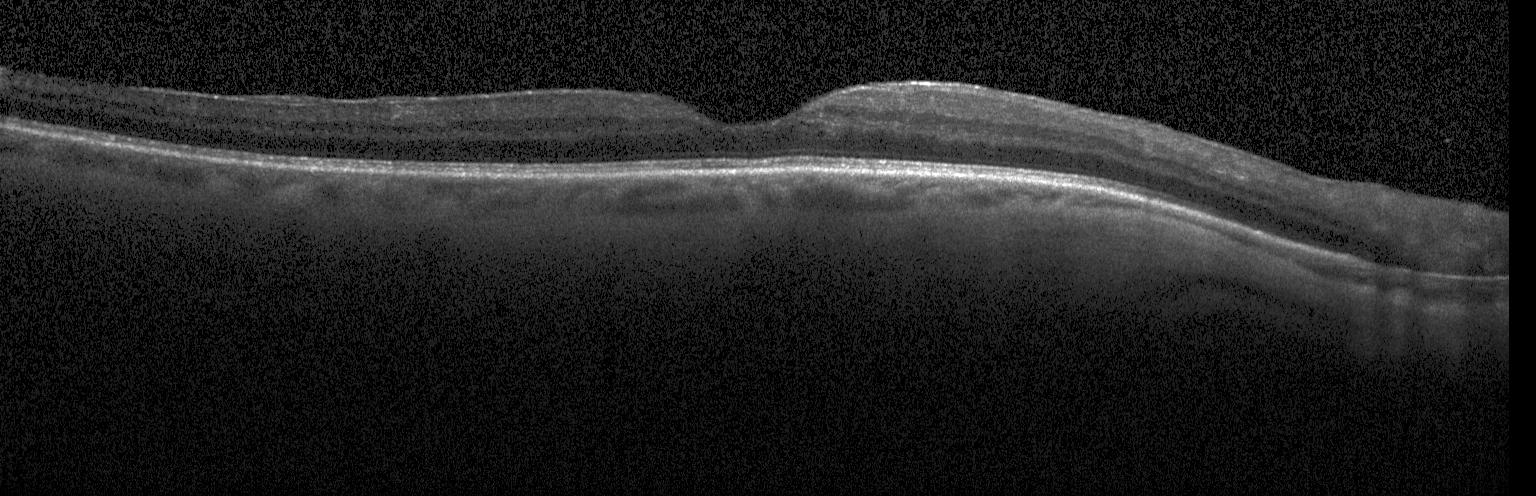 OCT line scan.
OCT finding: no CNV, DME, or drusen.